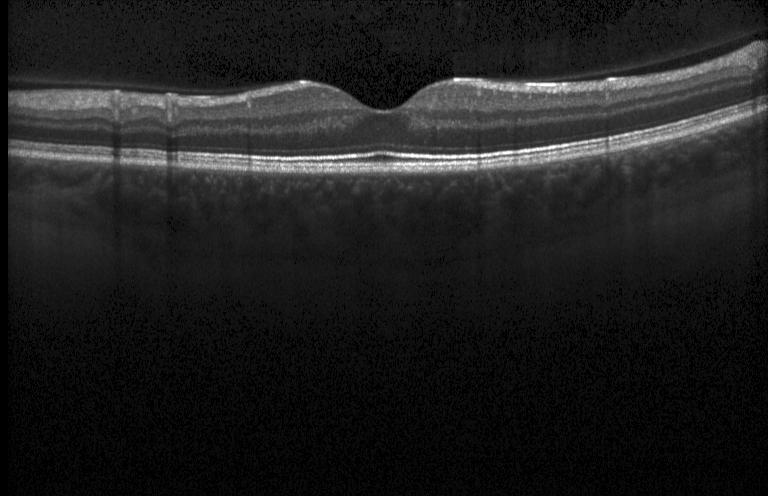
OCT finding: neither choroidal neovascularization, diabetic macular edema, nor drusen.